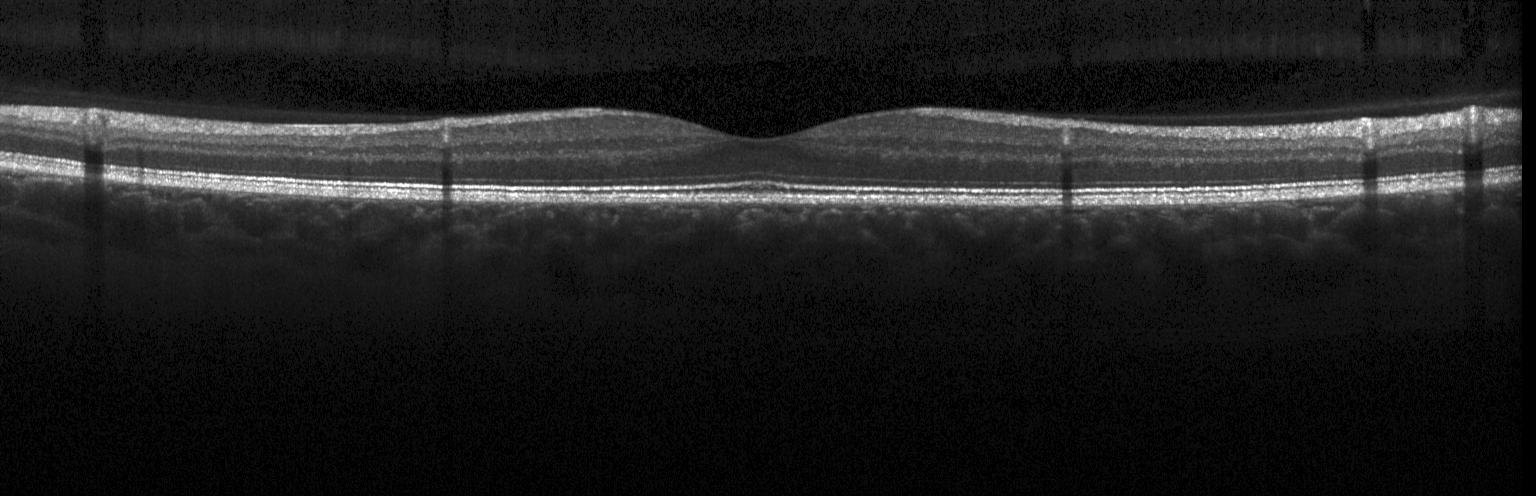

Spectral-domain optical coherence tomography · OCT B-scan · centered on the fovea. Impression: neither choroidal neovascularization, diabetic macular edema, nor drusen.